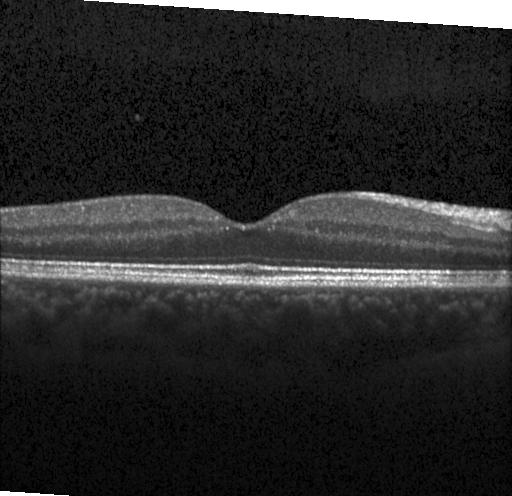
Spectral-domain OCT · Heidelberg Spectralis · fovea-centered · retinal OCT cross-section. Finding: no evidence of CNV, DME, or drusen.